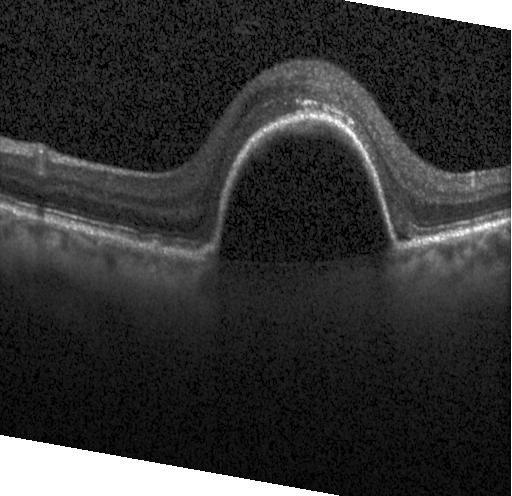 Retinal OCT B-scan. Assessment: choroidal neovascularization (CNV).